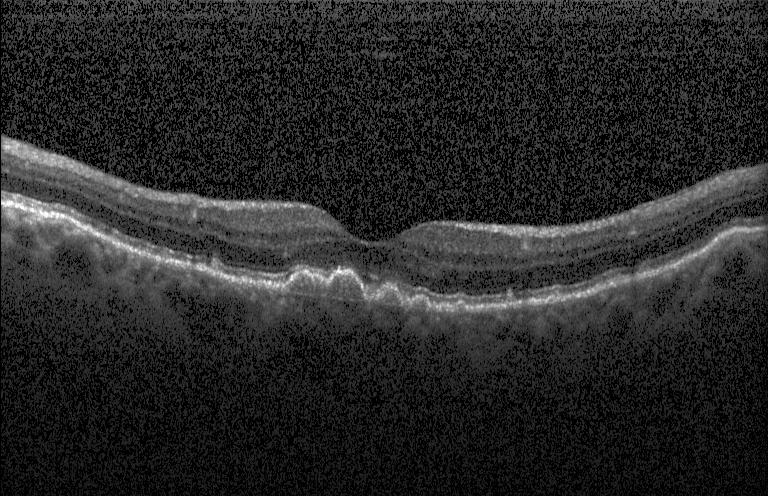

Spectral-domain OCT B-scan: sub-RPE drusenoid deposits.